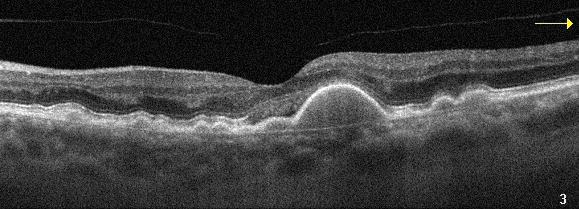 Retinal OCT B-scan
Diagnosis: AMD.